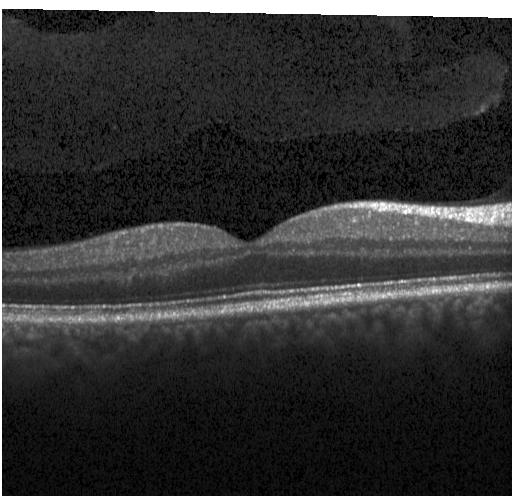

Optical coherence tomography scan; spectral-domain optical coherence tomography; macular scan — The scan shows neither choroidal neovascularization, diabetic macular edema, nor drusen.